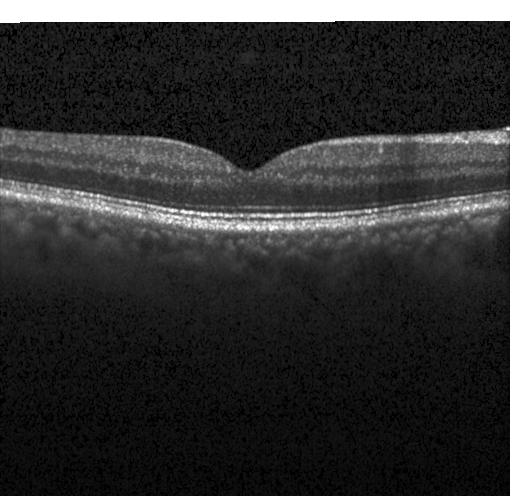

Instrument: Heidelberg Spectralis; SD-OCT; centered on the fovea; optical coherence tomography scan. The scan shows no CNV, no DME, and no drusen.